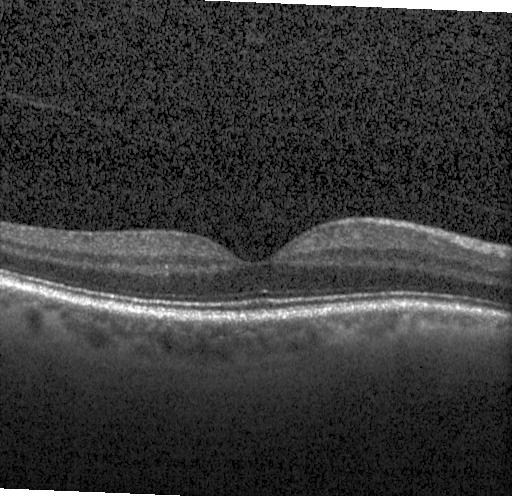
Macular OCT demonstrating no evidence of choroidal neovascularization, diabetic macular edema, or drusen.